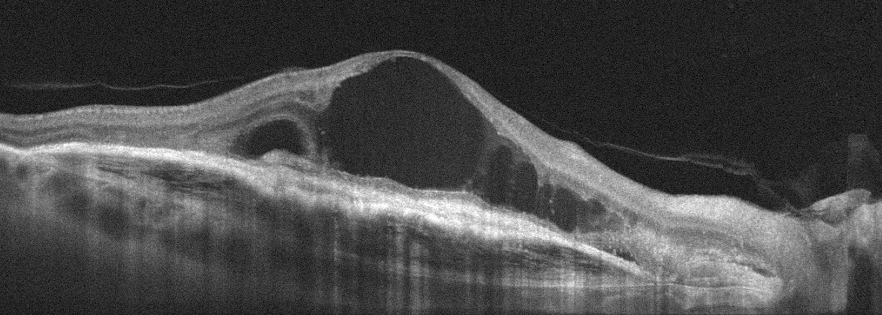
OD, retinal OCT B-scan.
Macular OCT: AMD.